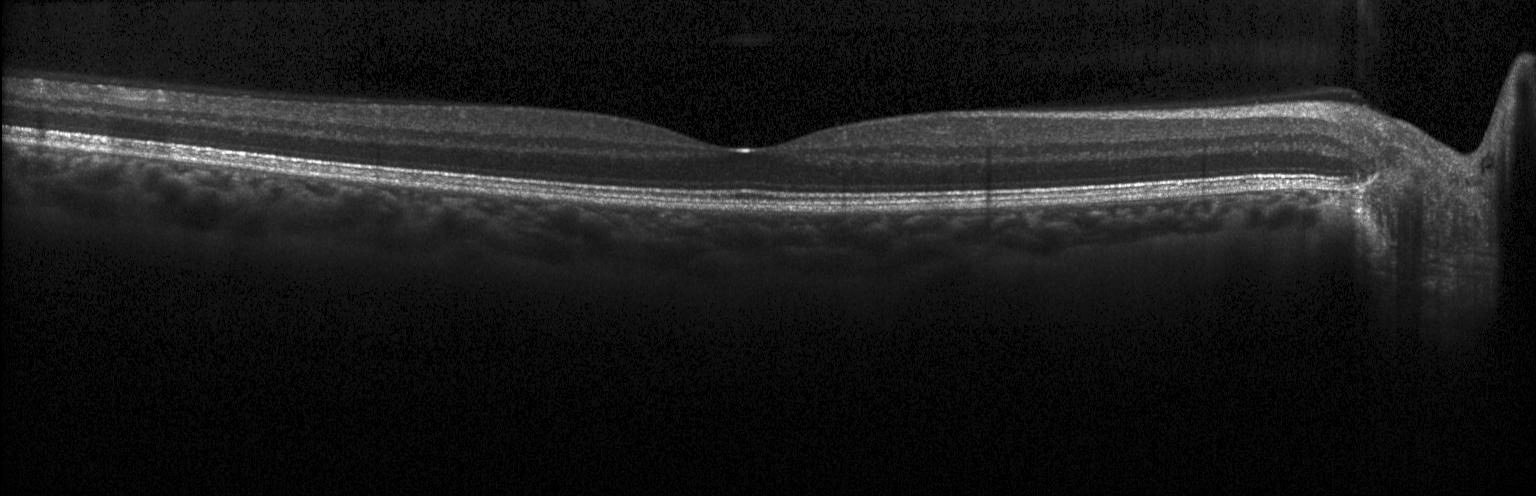
This B-scan demonstrates no choroidal neovascularization, diabetic macular edema, or drusen.